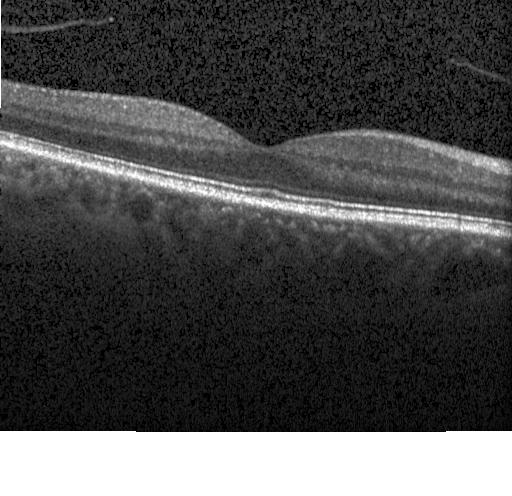 OCT finding: no choroidal neovascularization, diabetic macular edema, or drusen.